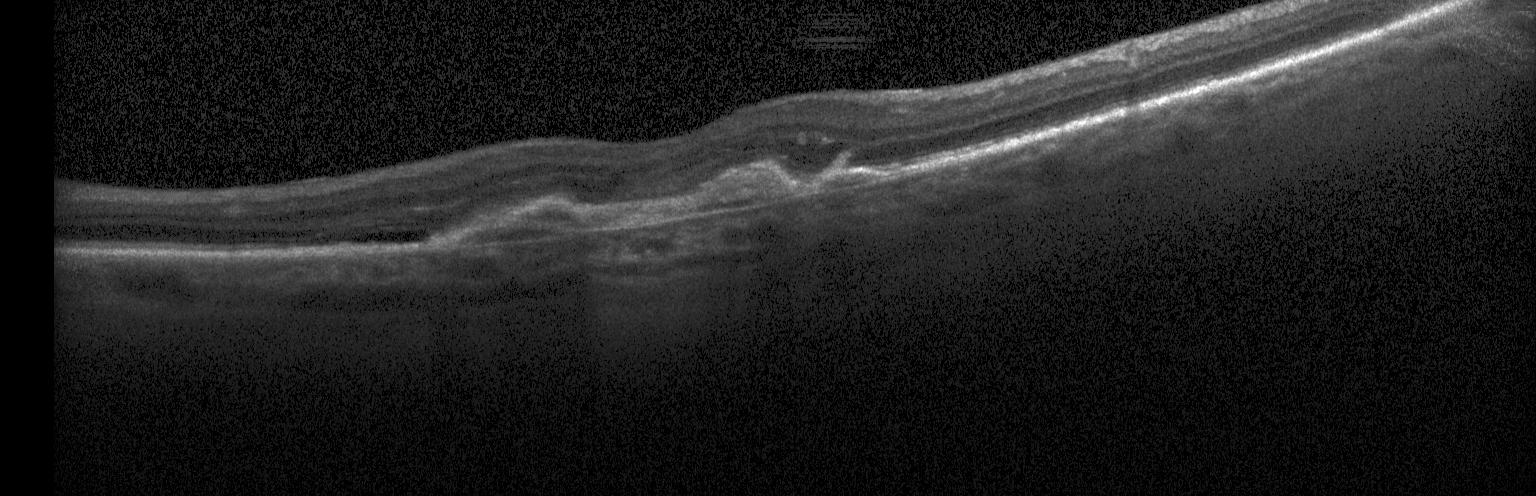 Finding: a choroidal neovascular membrane.